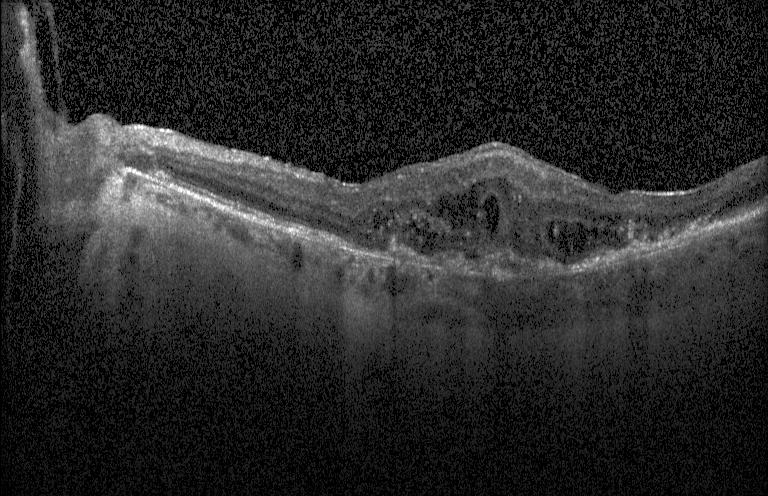

Retinal OCT B-scan. Fovea-centered. Instrument: Heidelberg Spectralis. Spectral-domain OCT. Diagnosis: a choroidal neovascular membrane.